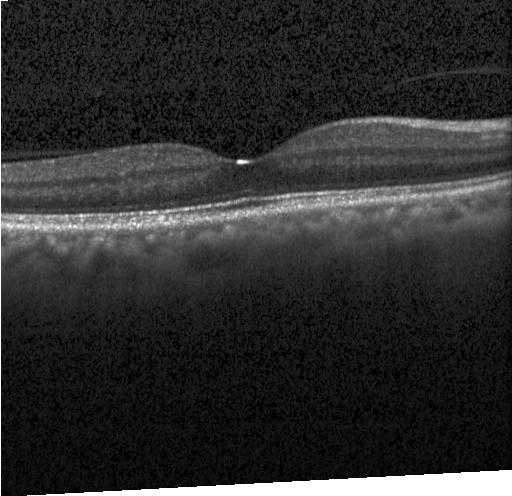
Optical coherence tomography scan.
This B-scan demonstrates no choroidal neovascularization, no diabetic macular edema, and no drusen.